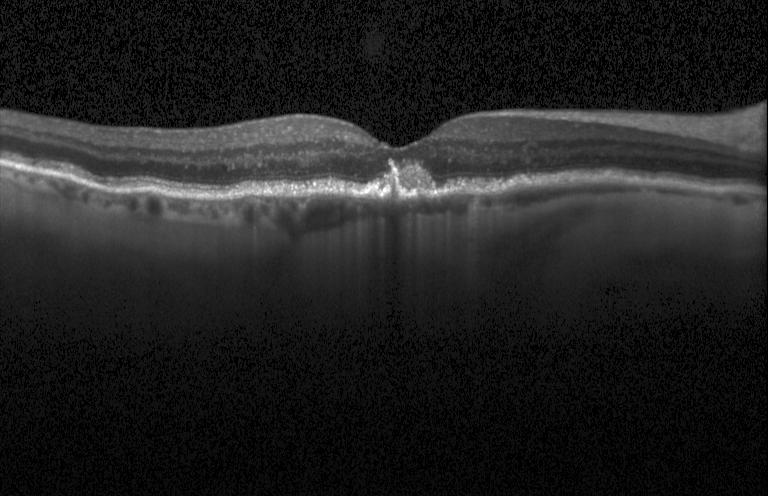
Retinal OCT B-scan. Through the macula. Heidelberg Spectralis OCT system.
Macular OCT: drusen.